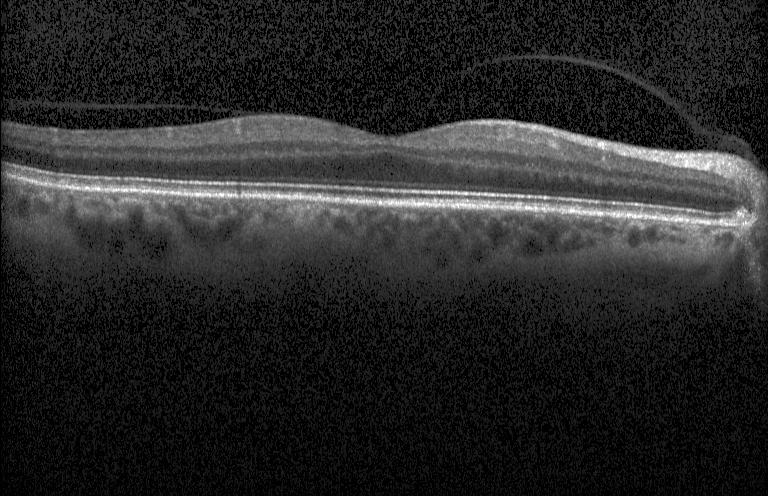

Spectral-domain OCT B-scan: no choroidal neovascularization, no diabetic macular edema, and no drusen.